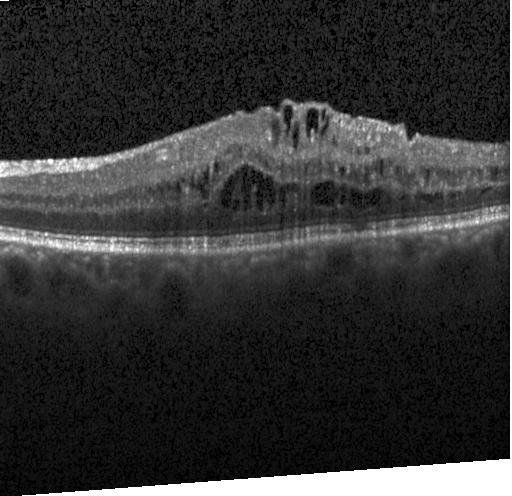
Acquired on a Heidelberg Spectralis · retinal OCT B-scan · horizontal scan through the fovea · spectral-domain OCT. Assessment: diabetic macular edema (DME).